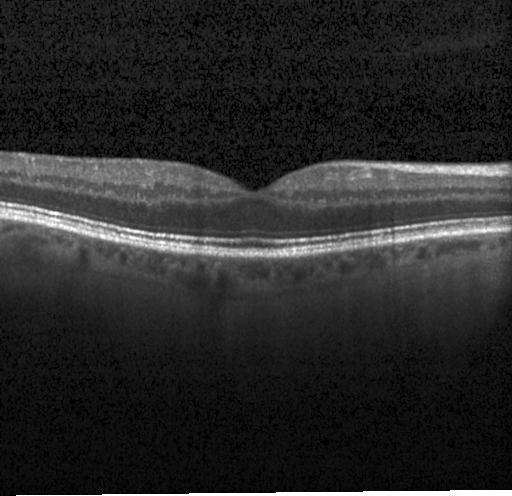

OCT B-scan.
The scan shows no evidence of choroidal neovascularization, diabetic macular edema, or drusen.